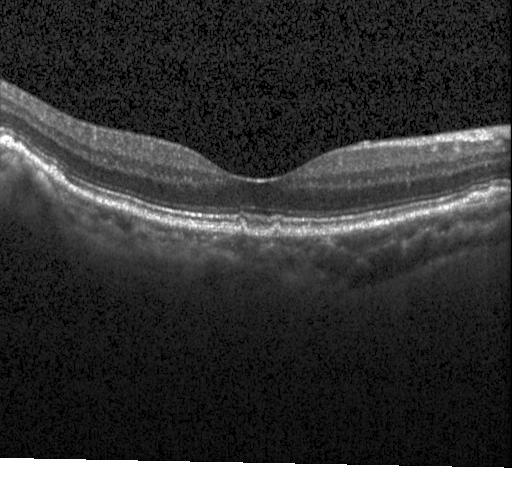

OCT scan showing drusen.